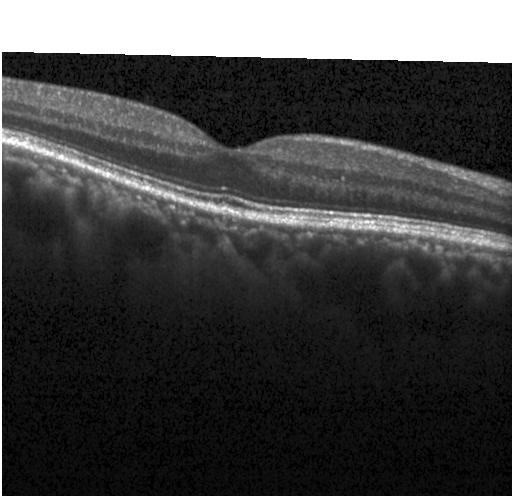
OCT finding: no evidence of choroidal neovascularization, diabetic macular edema, or drusen.